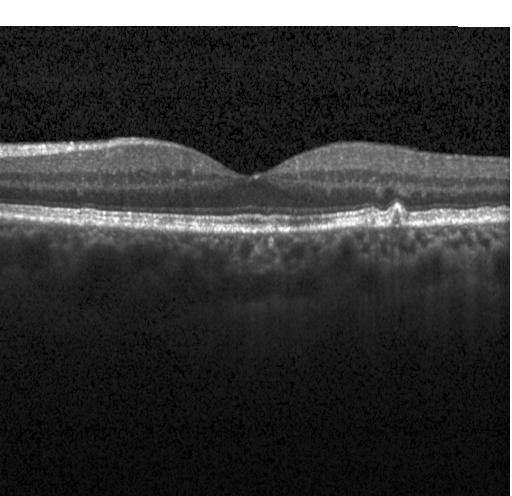
Optical coherence tomography B-scan — Dx: sub-RPE drusenoid deposits.